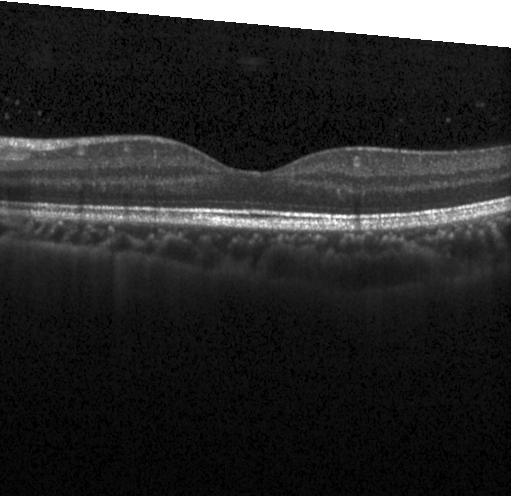
Acquired on a Heidelberg Spectralis; retinal OCT cross-section — Impression: no evidence of choroidal neovascularization, diabetic macular edema, or drusen.